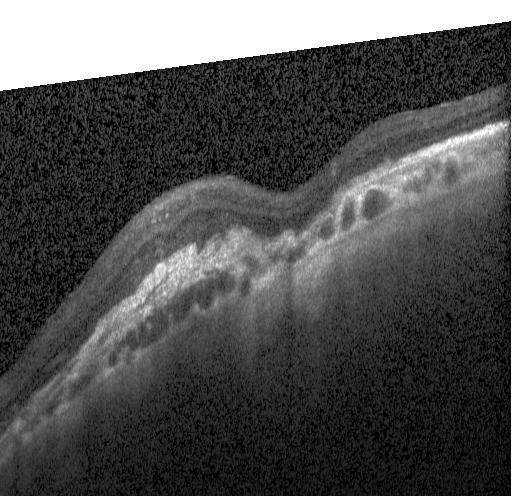 OCT B-scan showing a choroidal neovascular membrane.